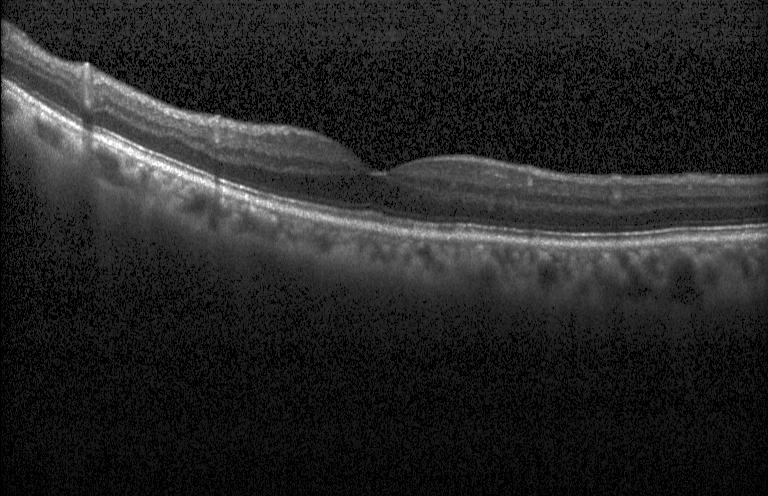

Retinal OCT cross-section, horizontal scan through the fovea, instrument: Heidelberg Spectralis — Diagnosis: no evidence of choroidal neovascularization, diabetic macular edema, or drusen.